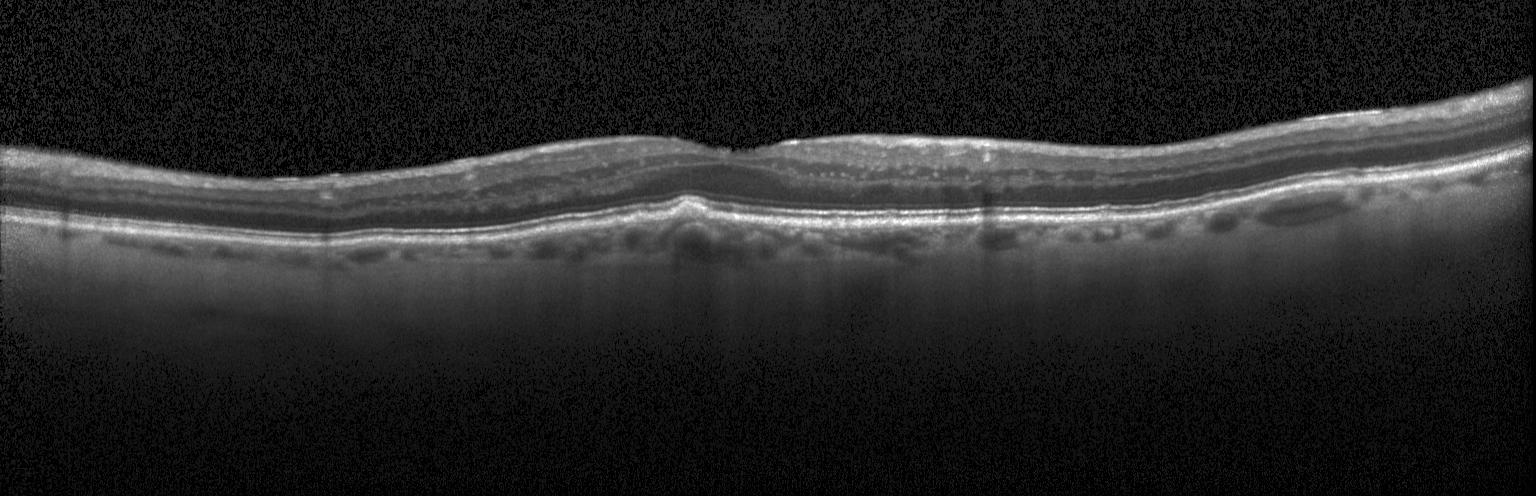

Instrument: Heidelberg Spectralis · retinal OCT B-scan · SD-OCT.
Diagnosis: sub-RPE drusenoid deposits.